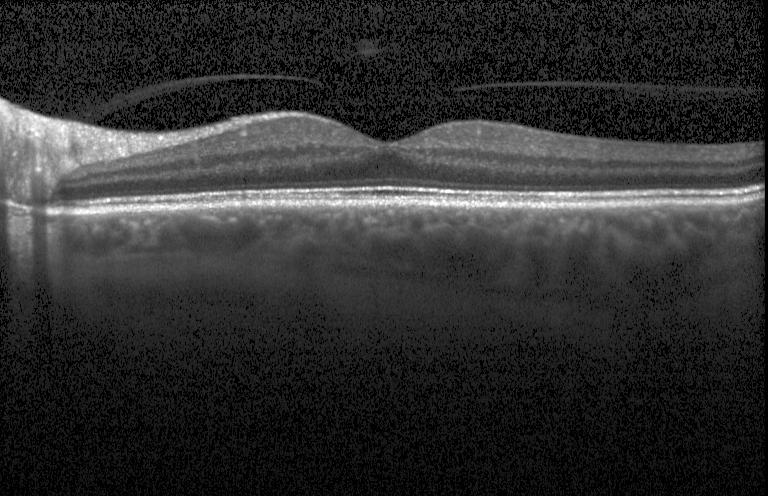

No CNV, DME, or drusen.